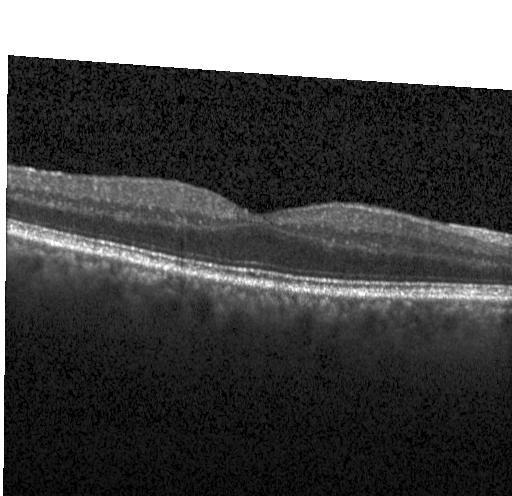

Retinal OCT cross-section.
Diagnosis: no evidence of choroidal neovascularization, diabetic macular edema, or drusen.